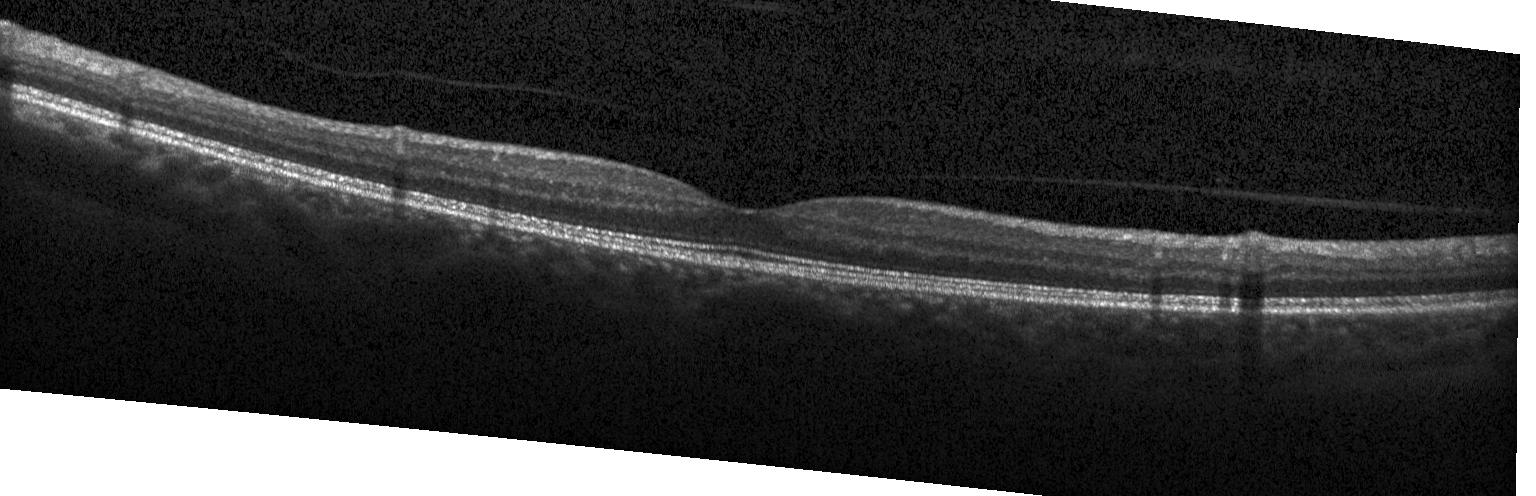 Diagnosis: no evidence of choroidal neovascularization, diabetic macular edema, or drusen.